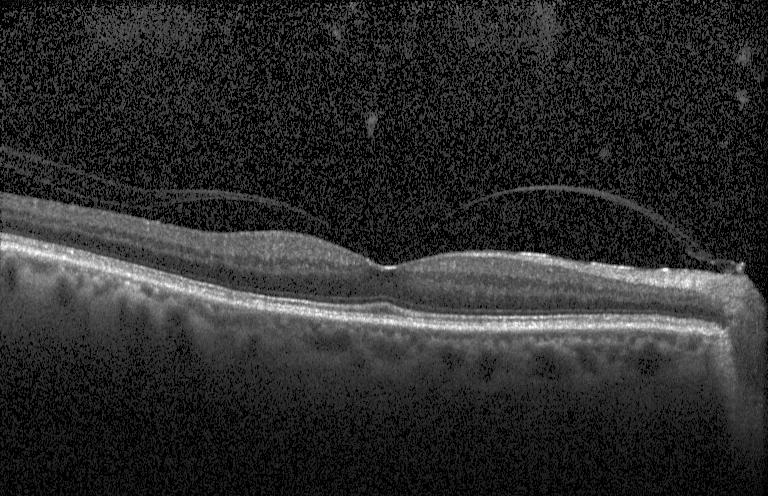 Optical coherence tomography B-scan. Acquired on a Heidelberg Spectralis. Horizontal scan through the fovea. Spectral-domain OCT.
Impression: no evidence of choroidal neovascularization, diabetic macular edema, or drusen.